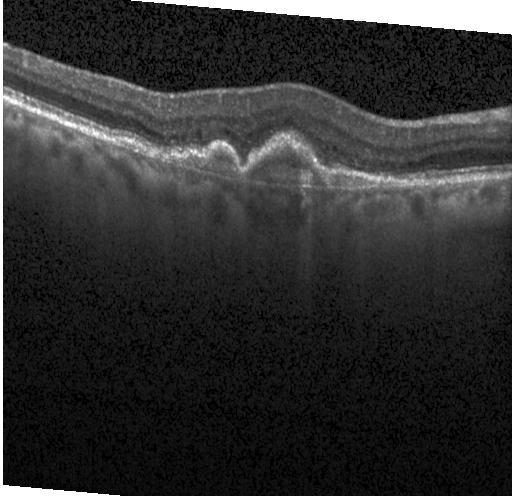

OCT finding: choroidal neovascularization (CNV).